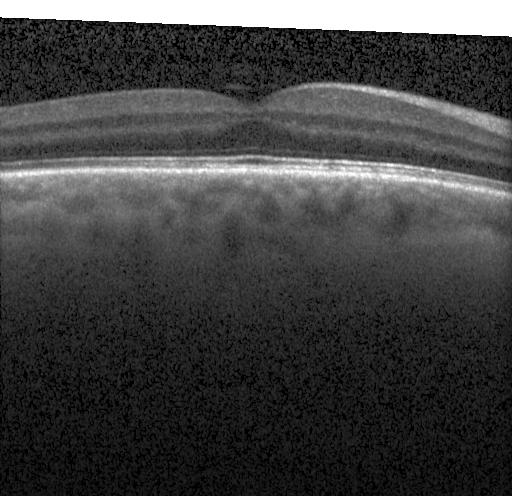

Macular scan, spectral-domain optical coherence tomography, OCT line scan, instrument: Heidelberg Spectralis. Impression: no choroidal neovascularization, diabetic macular edema, or drusen.